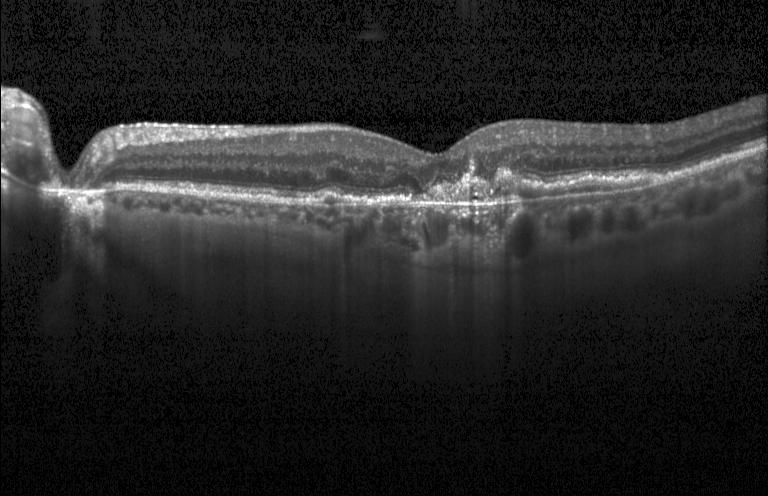 OCT line scan, spectral-domain OCT, fovea-centered. Assessment: choroidal neovascularization (CNV).